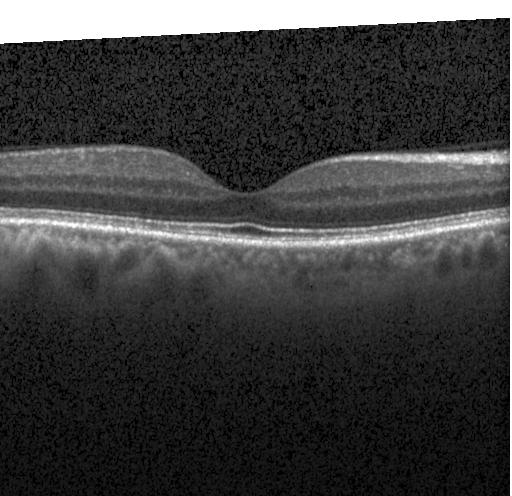 Spectral-domain OCT. Retinal OCT B-scan. Macular OCT: neither choroidal neovascularization, diabetic macular edema, nor drusen.